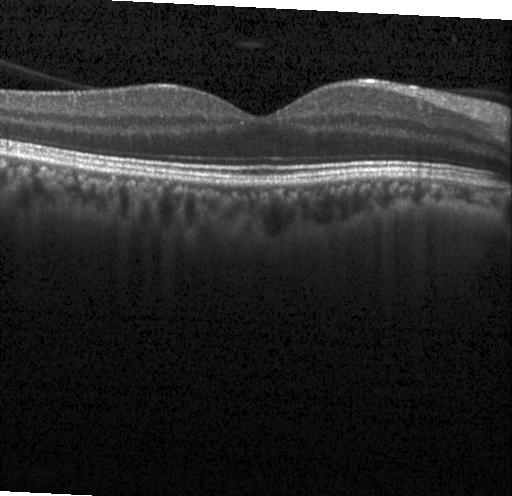

Through the macula; OCT line scan; spectral-domain optical coherence tomography. Finding: no evidence of choroidal neovascularization, diabetic macular edema, or drusen.